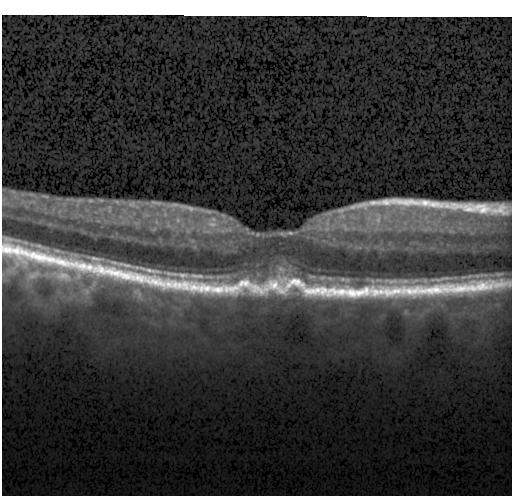
Assessment: drusen.